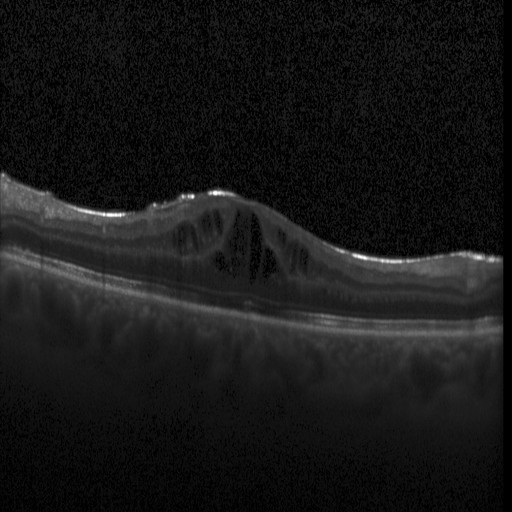

Centered on the fovea; OCT B-scan.
Finding: diabetic macular edema.